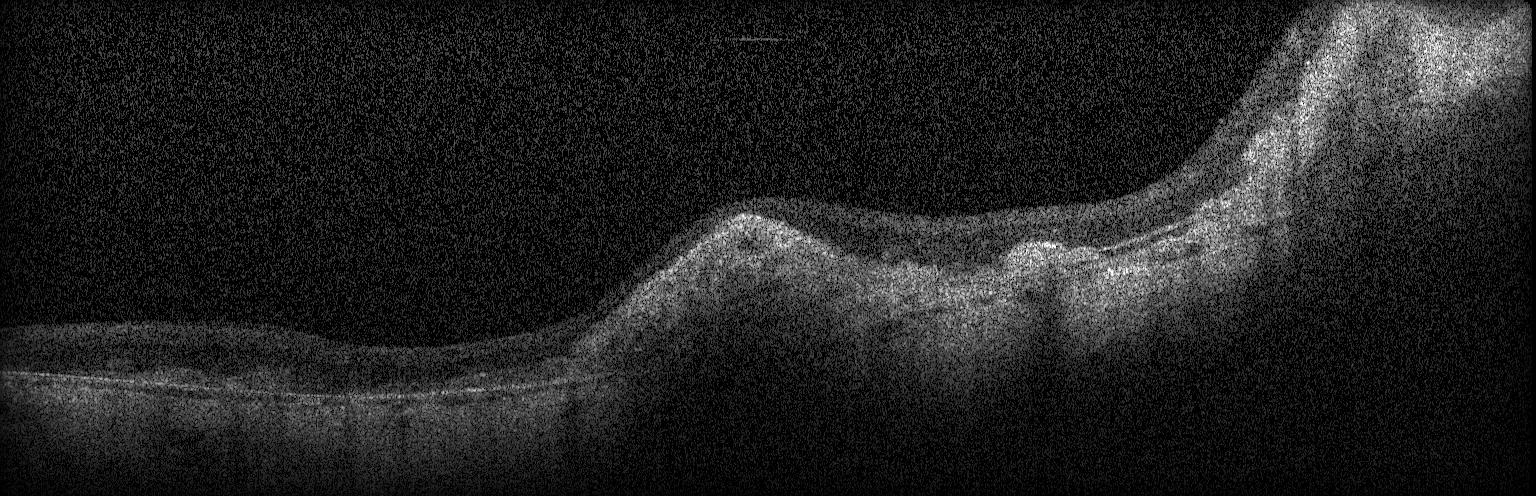
Diagnosis: a choroidal neovascular membrane.